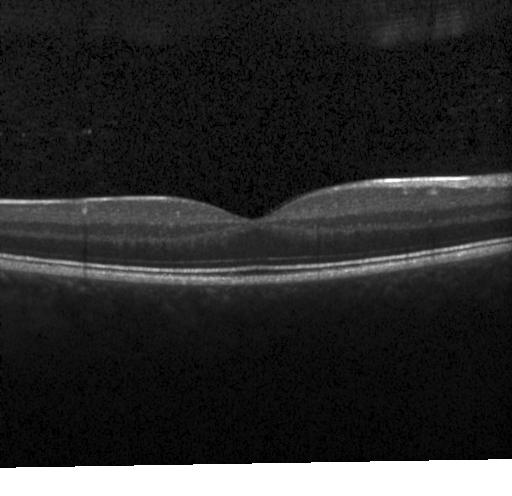

This B-scan demonstrates no choroidal neovascularization, diabetic macular edema, or drusen.